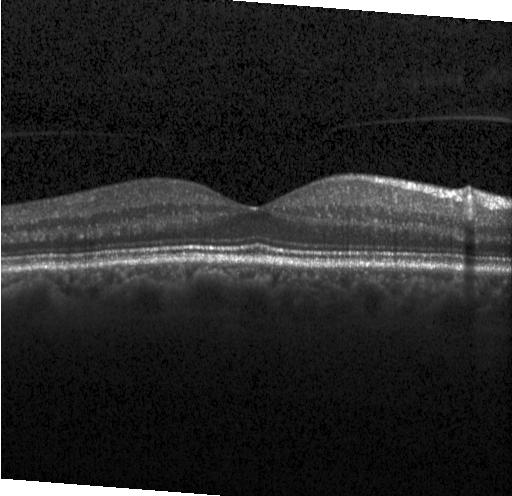
Optical coherence tomography scan, Heidelberg Spectralis.
Finding: no evidence of CNV, DME, or drusen.